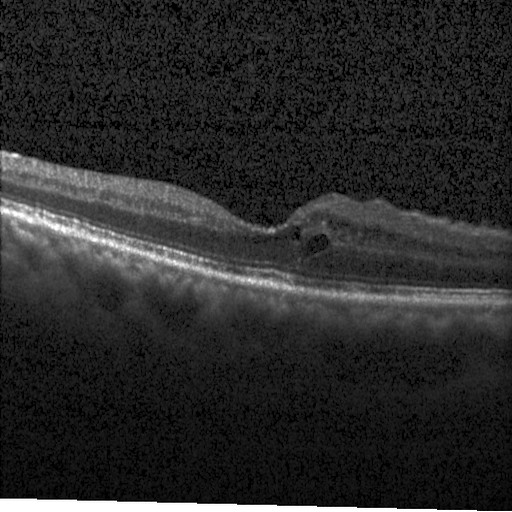 Heidelberg Spectralis OCT system; optical coherence tomography B-scan. This B-scan demonstrates diabetic macular edema (DME).